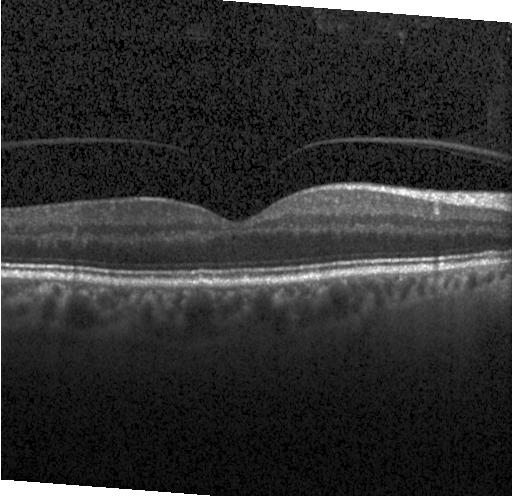
Centered on the fovea; spectral-domain optical coherence tomography; OCT B-scan.
Finding: no evidence of choroidal neovascularization, diabetic macular edema, or drusen.